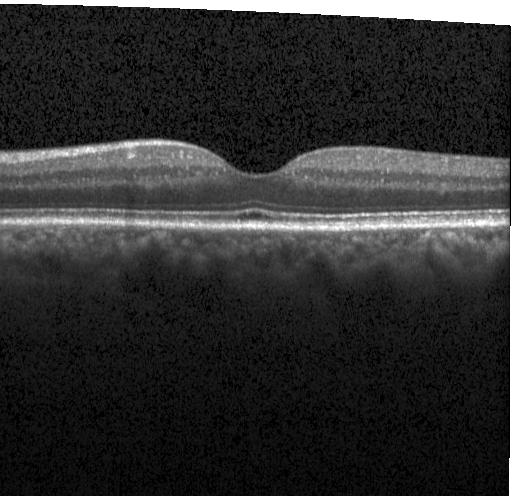
Dx: neither CNV, DME, nor drusen.